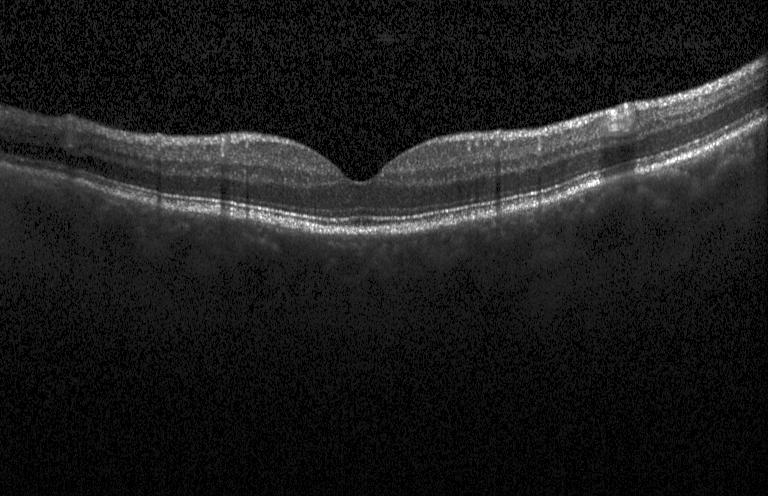 Instrument: Heidelberg Spectralis · optical coherence tomography B-scan · macular scan.
Dx: no choroidal neovascularization, diabetic macular edema, or drusen.